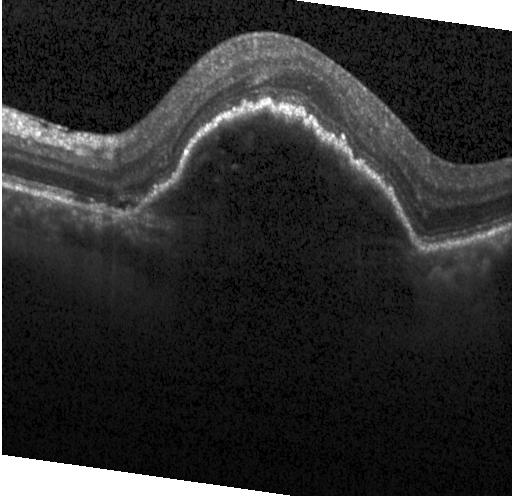

Retinal OCT cross-section.
OCT finding: a choroidal neovascular membrane.